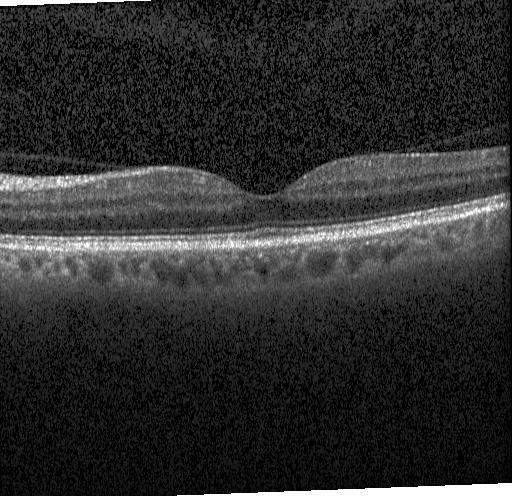 This B-scan demonstrates no evidence of choroidal neovascularization, diabetic macular edema, or drusen.